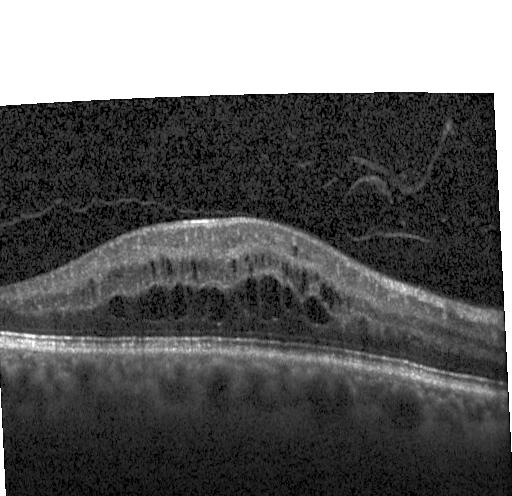

Optical coherence tomography B-scan.
Diabetic macular edema (DME).